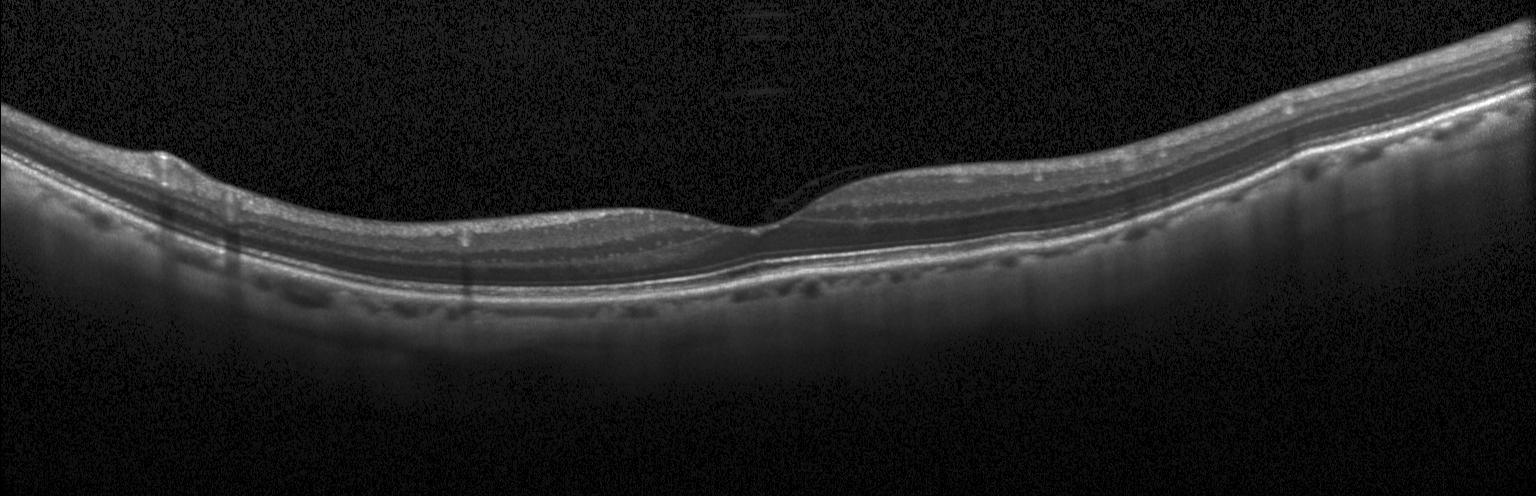 Macular OCT demonstrating no CNV, no DME, and no drusen.